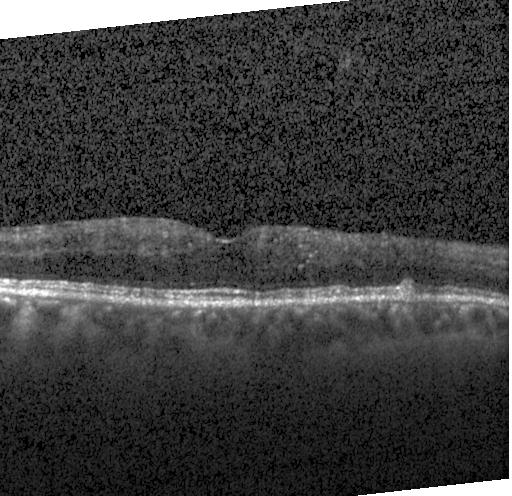

Acquired on a Heidelberg Spectralis. Retinal OCT cross-section. Horizontal scan through the fovea. Spectral-domain optical coherence tomography. Finding: diabetic macular edema.